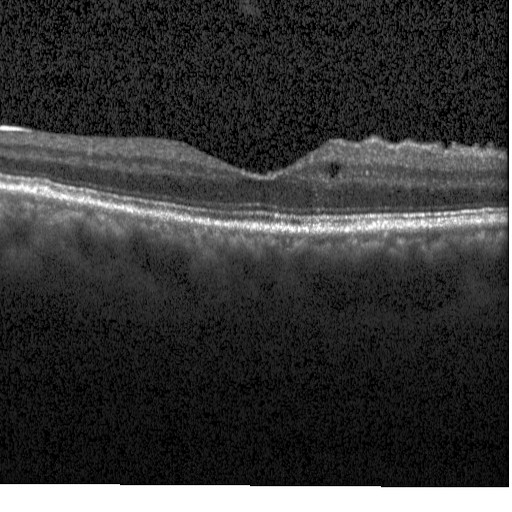
Diabetic macular edema.